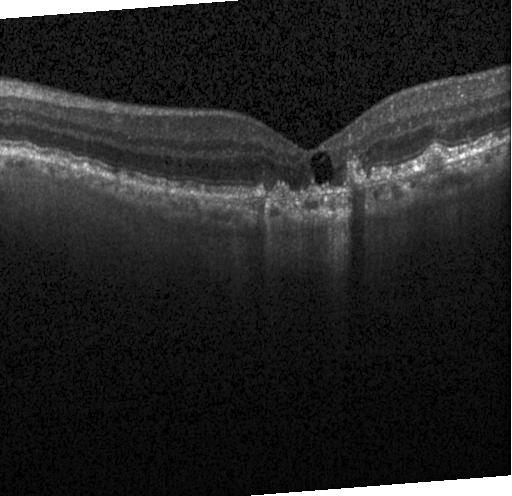 Retinal OCT B-scan. The scan shows a choroidal neovascular membrane.